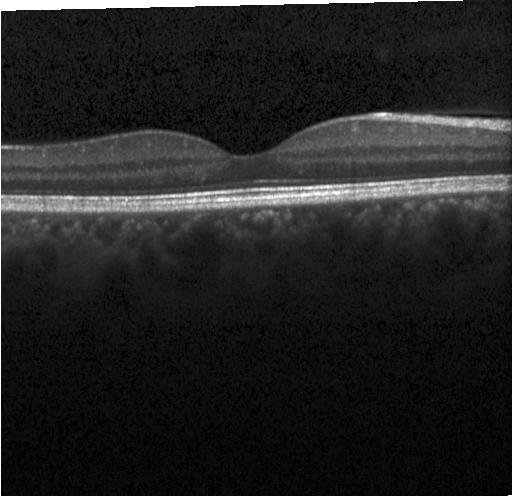 OCT B-scan. No choroidal neovascularization, diabetic macular edema, or drusen.